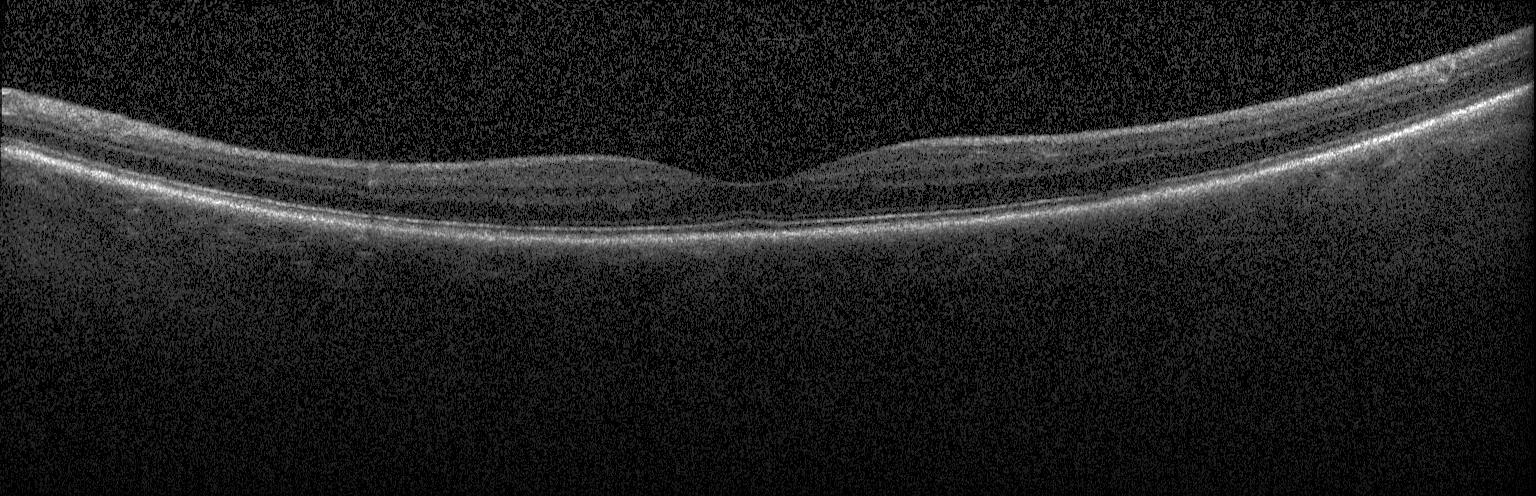
Retinal OCT B-scan. Fovea-centered — No evidence of choroidal neovascularization, diabetic macular edema, or drusen.